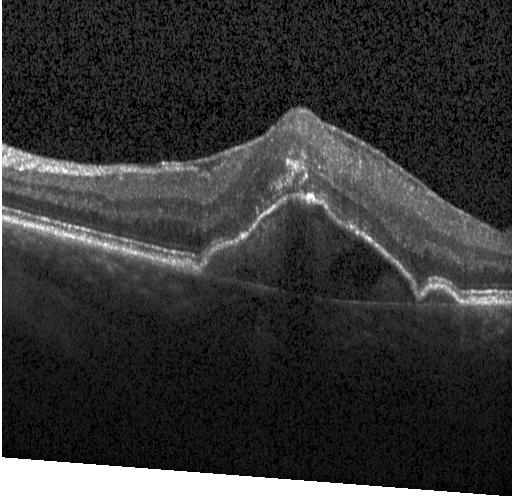
Acquired on a Heidelberg Spectralis. SD-OCT. OCT line scan
Impression: a choroidal neovascular membrane.